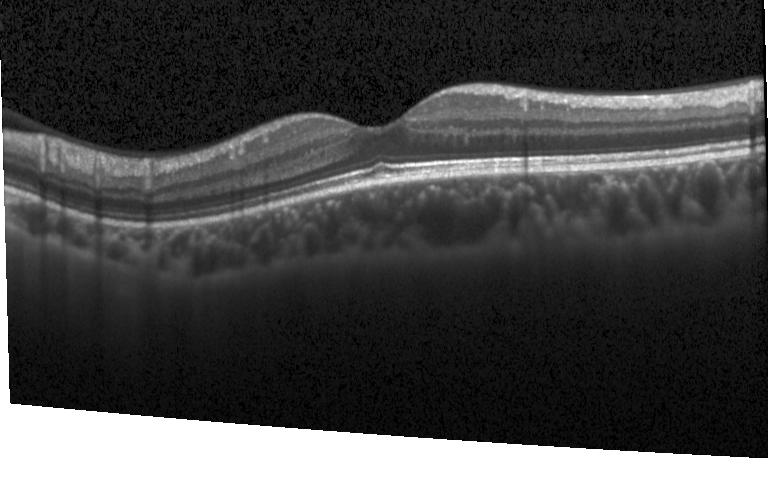 Optical coherence tomography B-scan, fovea-centered.
No CNV, no DME, and no drusen.